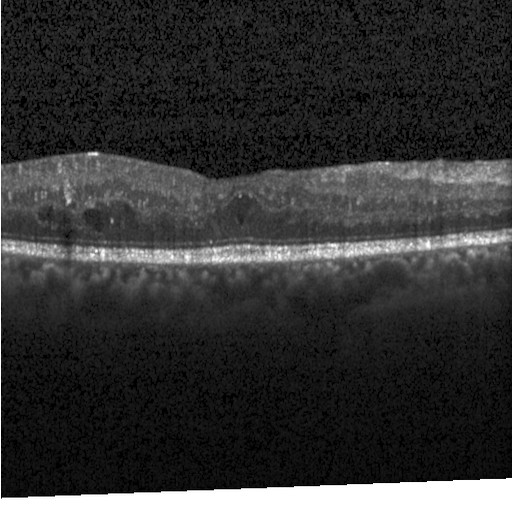

Dx: DME.